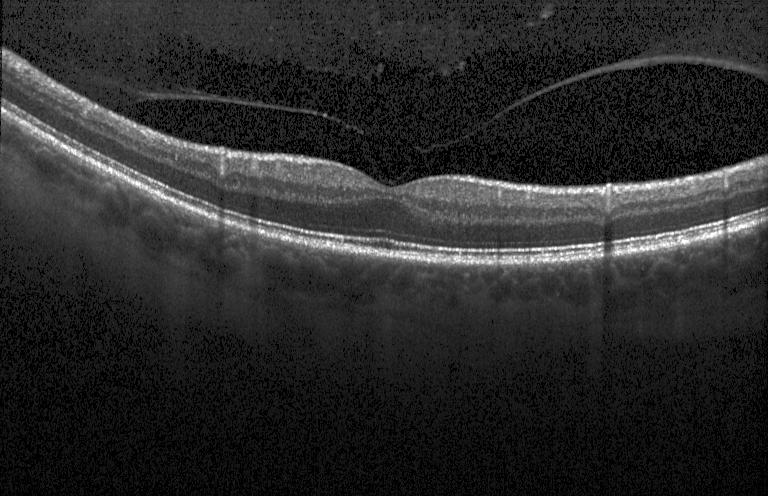
OCT line scan · fovea-centered — Finding: neither CNV, DME, nor drusen.